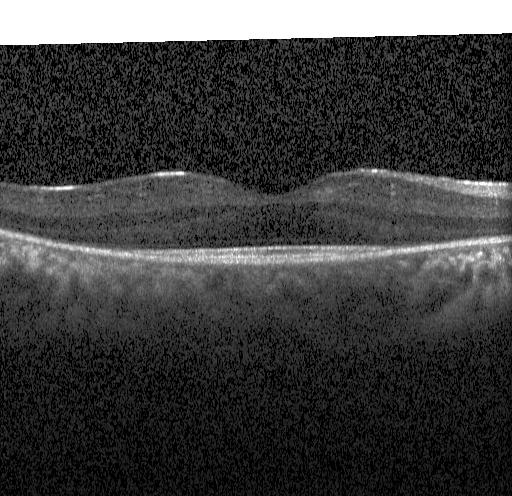

Macular OCT: neither choroidal neovascularization, diabetic macular edema, nor drusen.